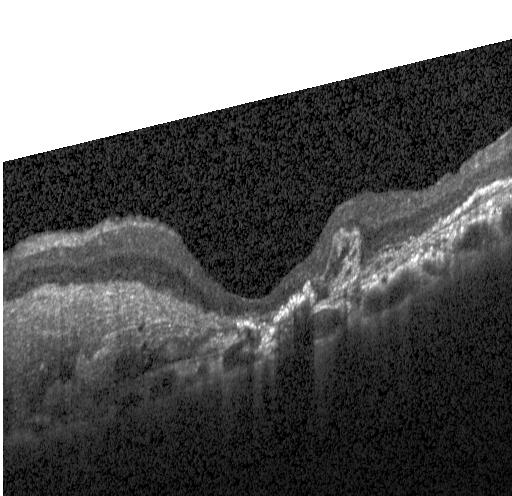
Heidelberg Spectralis · optical coherence tomography scan · fovea-centered · spectral-domain OCT — The scan shows choroidal neovascularization.